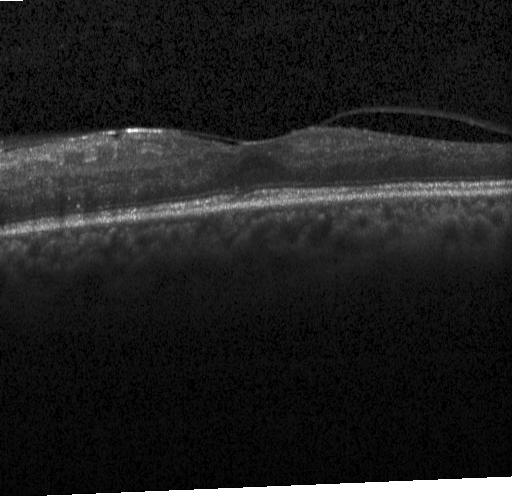 Impression: diabetic macular edema (DME).